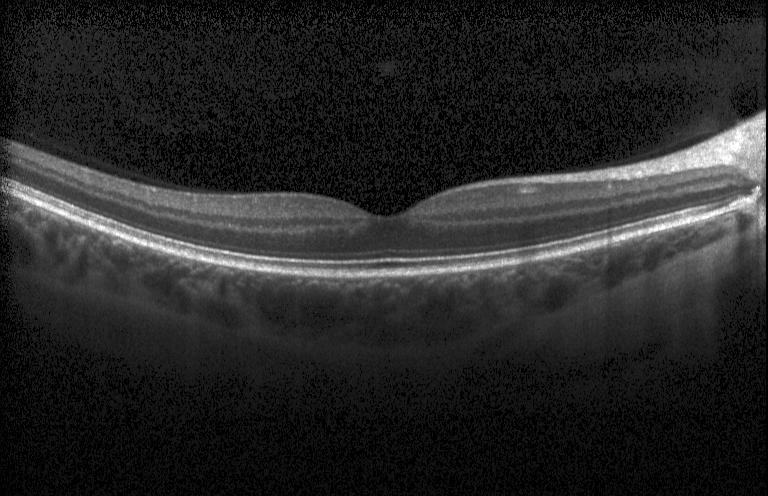 Acquired on a Heidelberg Spectralis. OCT B-scan. Horizontal scan through the fovea — No evidence of choroidal neovascularization, diabetic macular edema, or drusen.